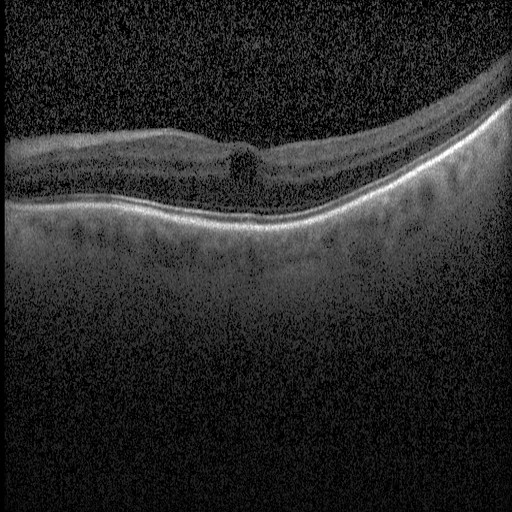 Instrument: Heidelberg Spectralis, spectral-domain OCT, optical coherence tomography B-scan, through the macula
This B-scan demonstrates DME.